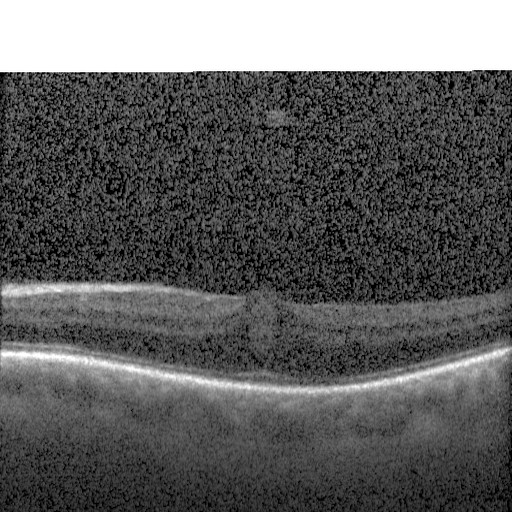
Finding: diabetic macular edema (DME).